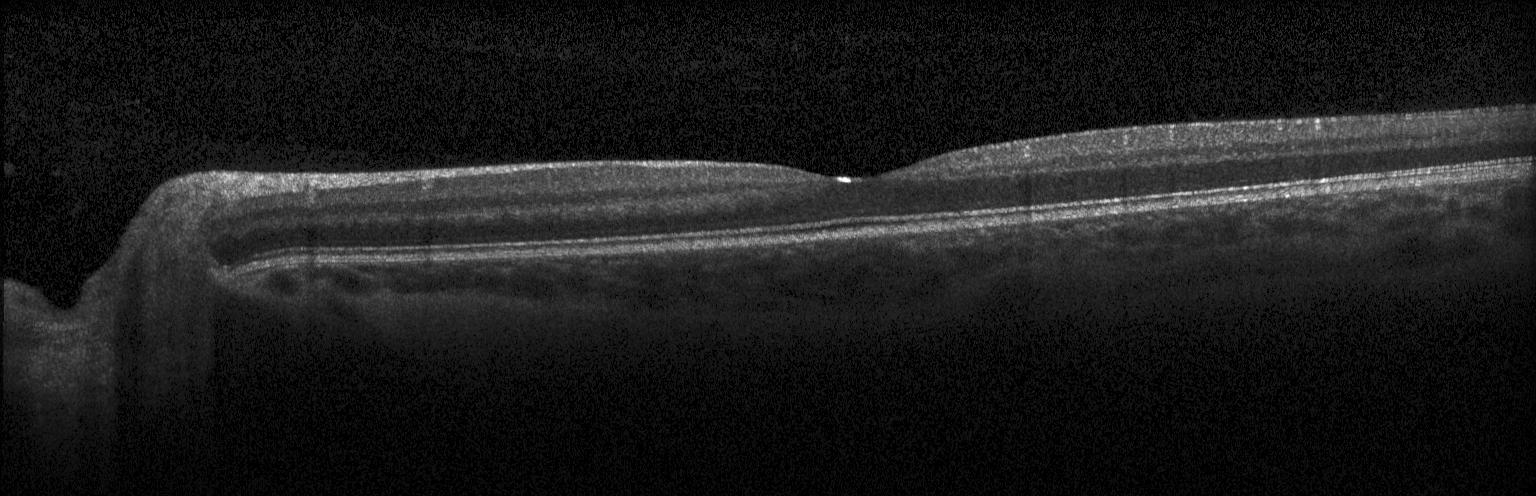
Macular OCT demonstrating no choroidal neovascularization, diabetic macular edema, or drusen.